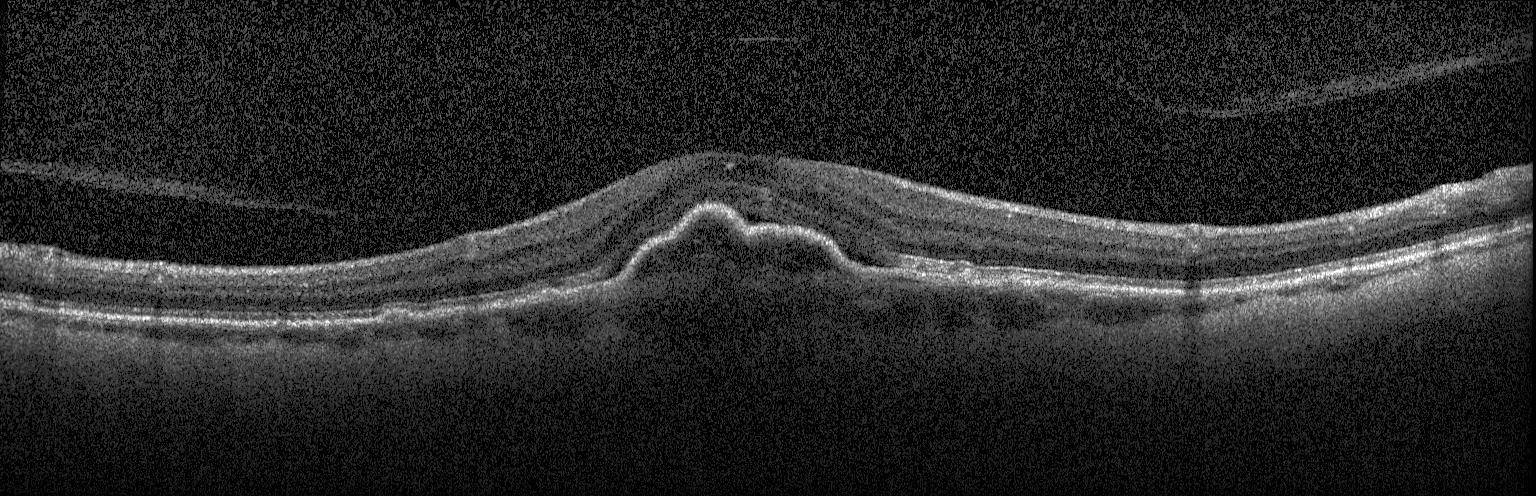

OCT finding: a choroidal neovascular membrane.